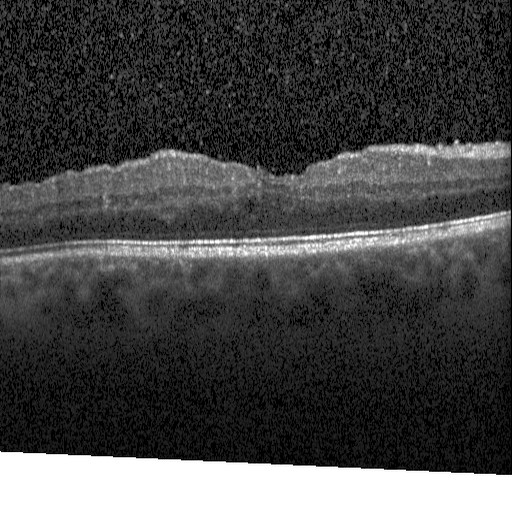
Optical coherence tomography scan
This B-scan demonstrates diabetic macular edema.